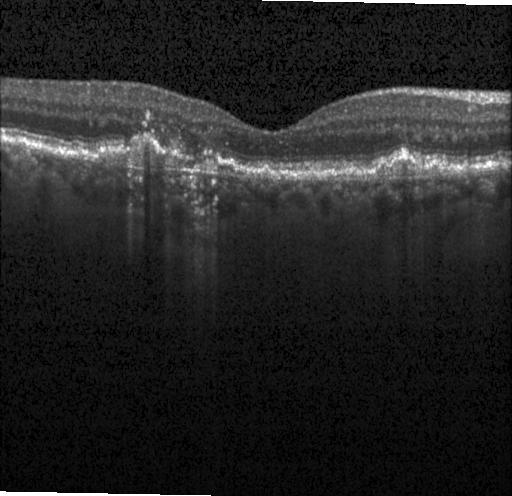 Heidelberg Spectralis OCT system. OCT line scan. SD-OCT. Fovea-centered. This B-scan demonstrates a choroidal neovascular membrane.